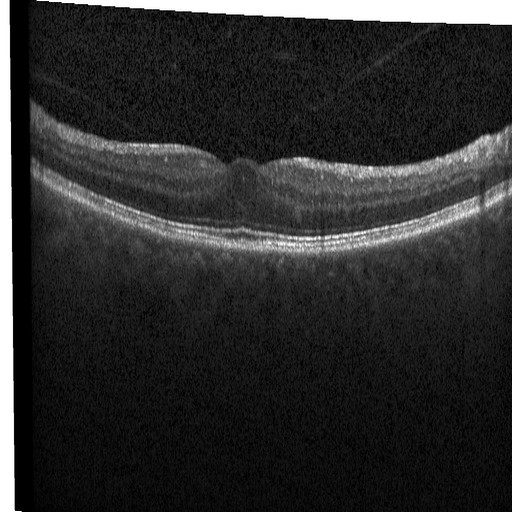

Retinal OCT cross-section
OCT finding: diabetic macular edema.